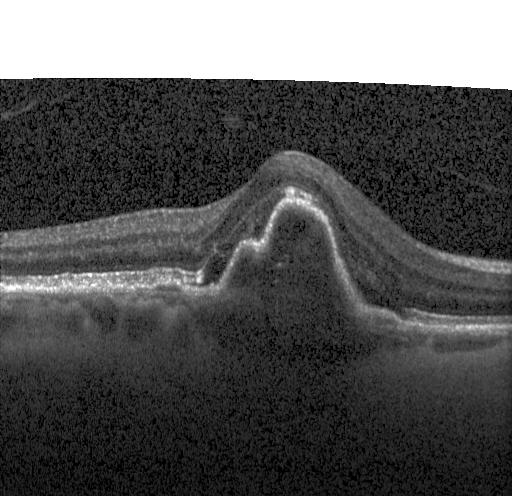 Horizontal scan through the fovea. SD-OCT. Optical coherence tomography scan
A choroidal neovascular membrane.